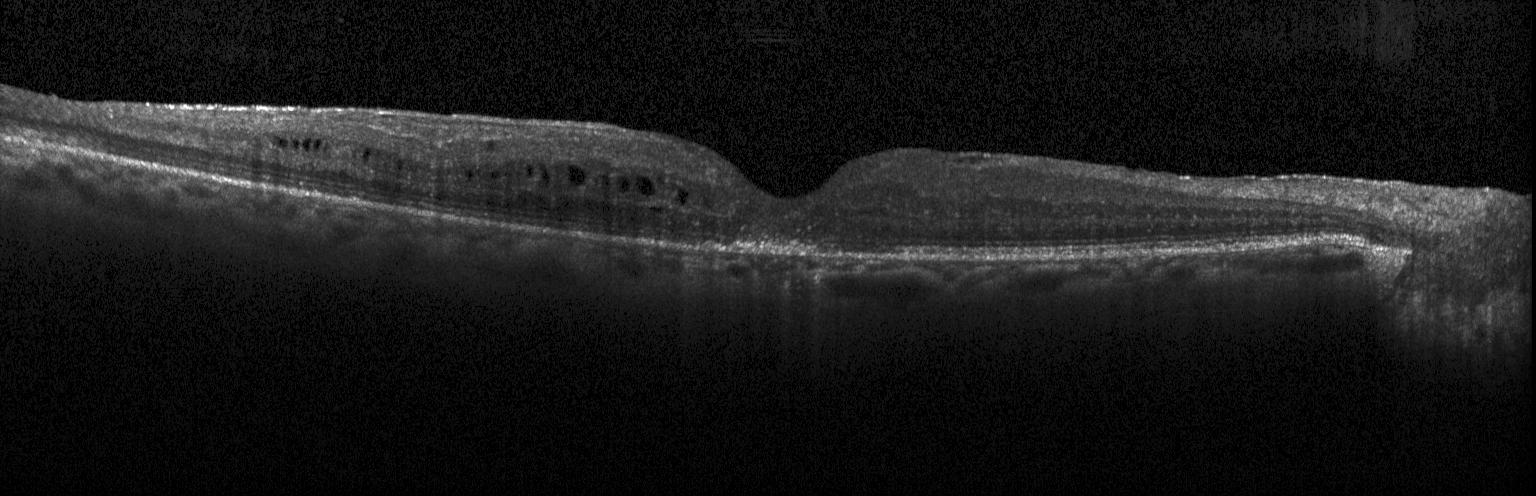 Retinal OCT B-scan. Horizontal scan through the fovea. Spectral-domain optical coherence tomography. Instrument: Heidelberg Spectralis.
This B-scan demonstrates DME.